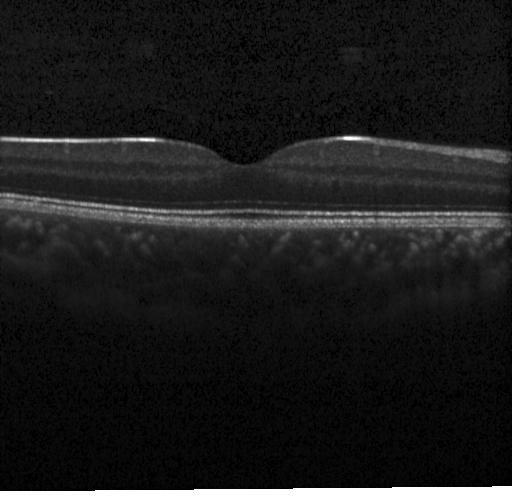

Finding: no CNV, no DME, and no drusen.